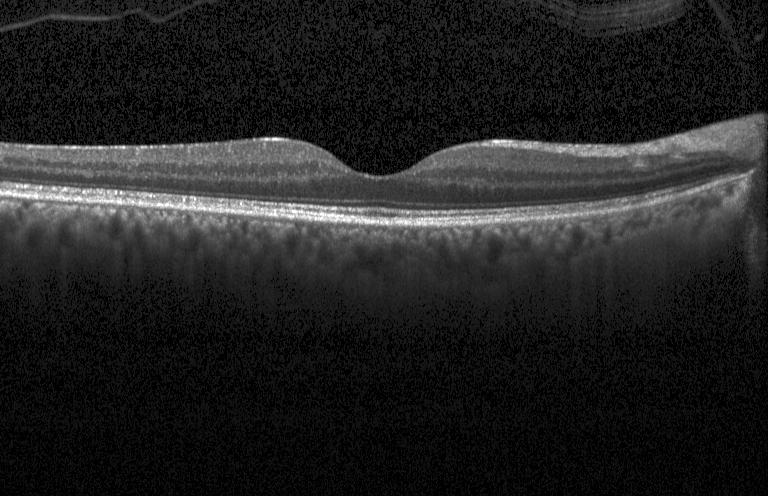

Retinal OCT cross-section, Heidelberg Spectralis, through the macula.
This B-scan demonstrates no CNV, no DME, and no drusen.